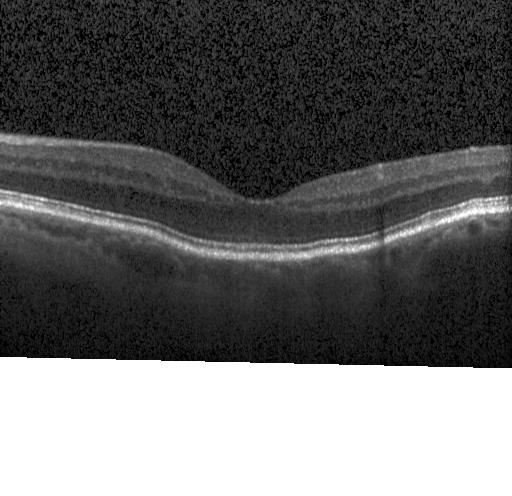

Spectral-domain OCT · optical coherence tomography B-scan · Heidelberg Spectralis · fovea-centered. Assessment: no choroidal neovascularization, diabetic macular edema, or drusen.